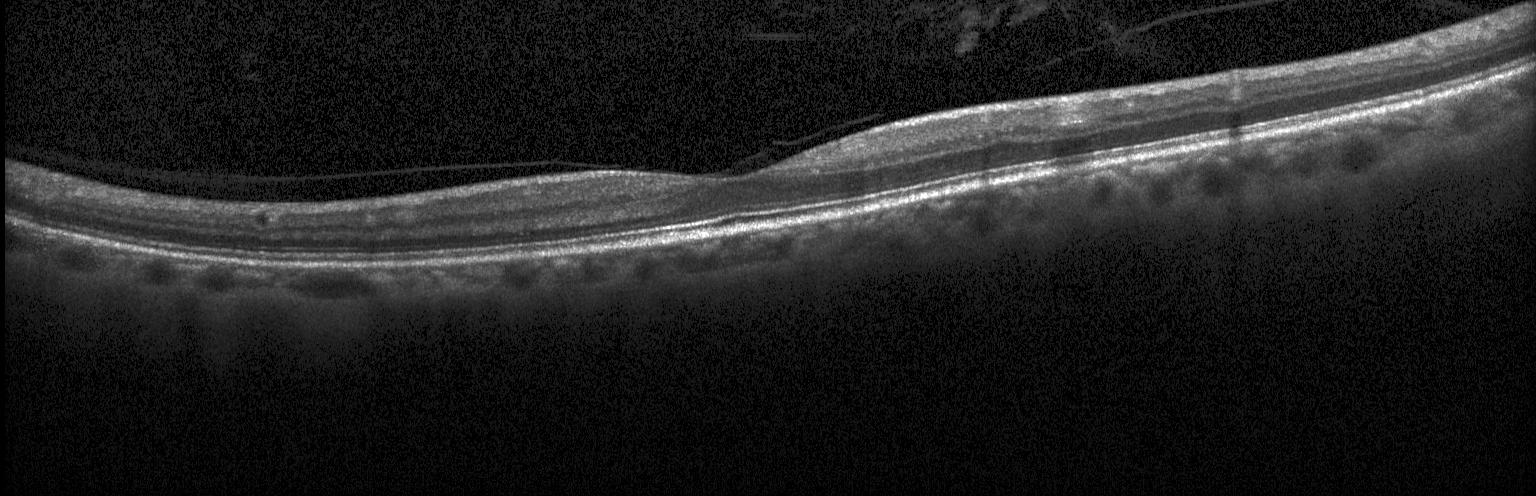 Diagnosis: neither CNV, DME, nor drusen.